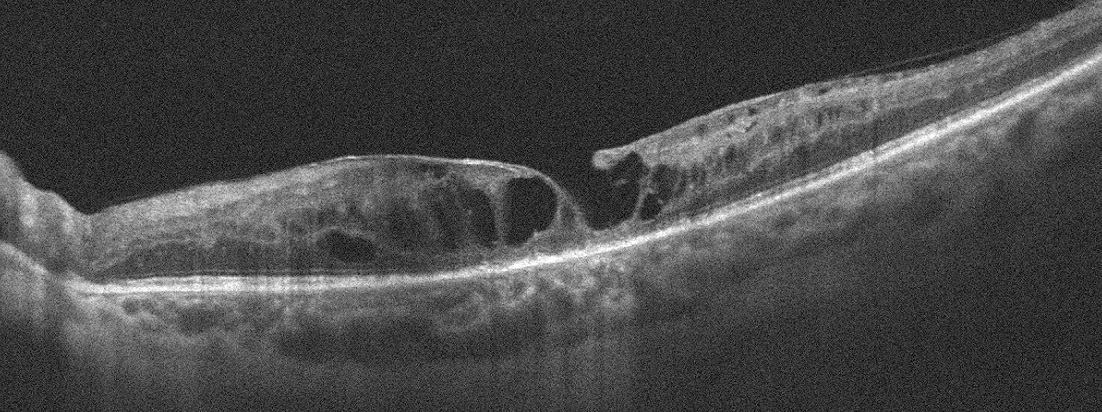

Finding: DME.